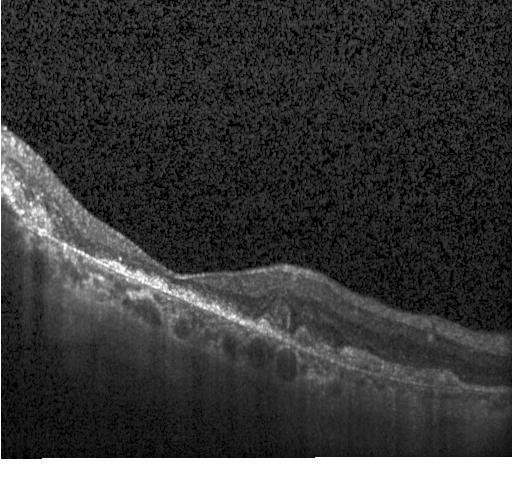

Spectral-domain optical coherence tomography, OCT B-scan. Dx: choroidal neovascularization (CNV).